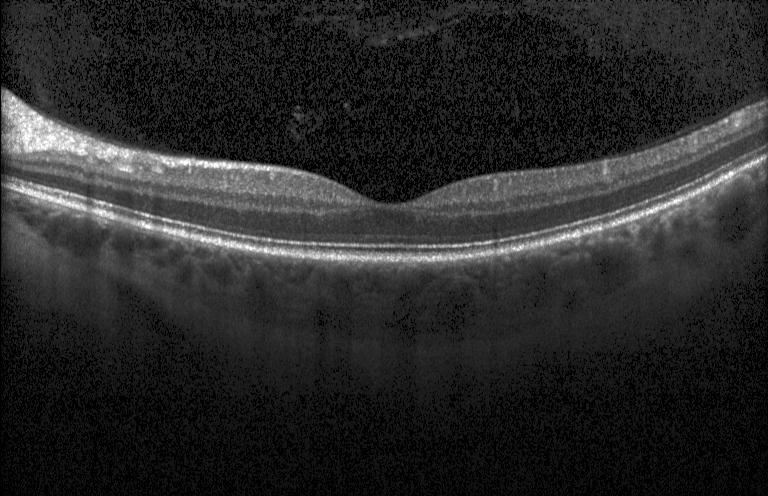 Spectral-domain optical coherence tomography · retinal OCT cross-section
Dx: no evidence of choroidal neovascularization, diabetic macular edema, or drusen.